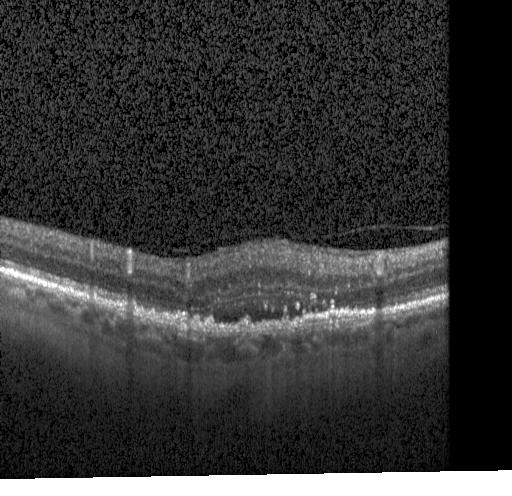 OCT B-scan.
Assessment: a choroidal neovascular membrane.